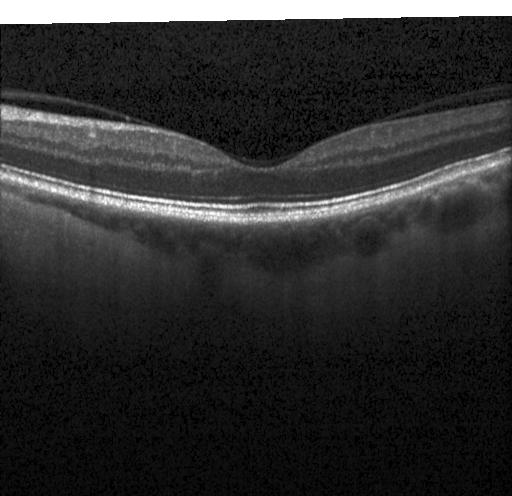 Horizontal scan through the fovea, retinal OCT B-scan — Finding: no evidence of CNV, DME, or drusen.